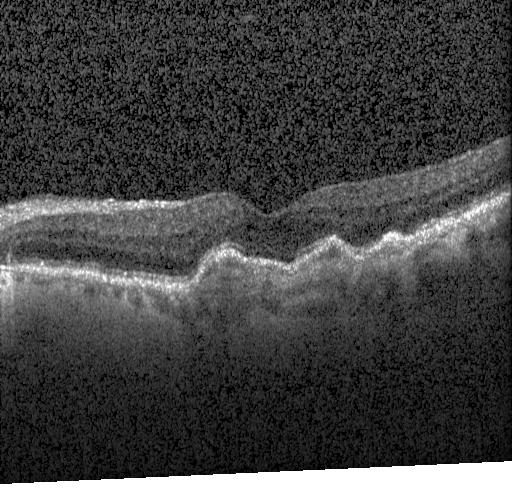

Diagnosis: a choroidal neovascular membrane.